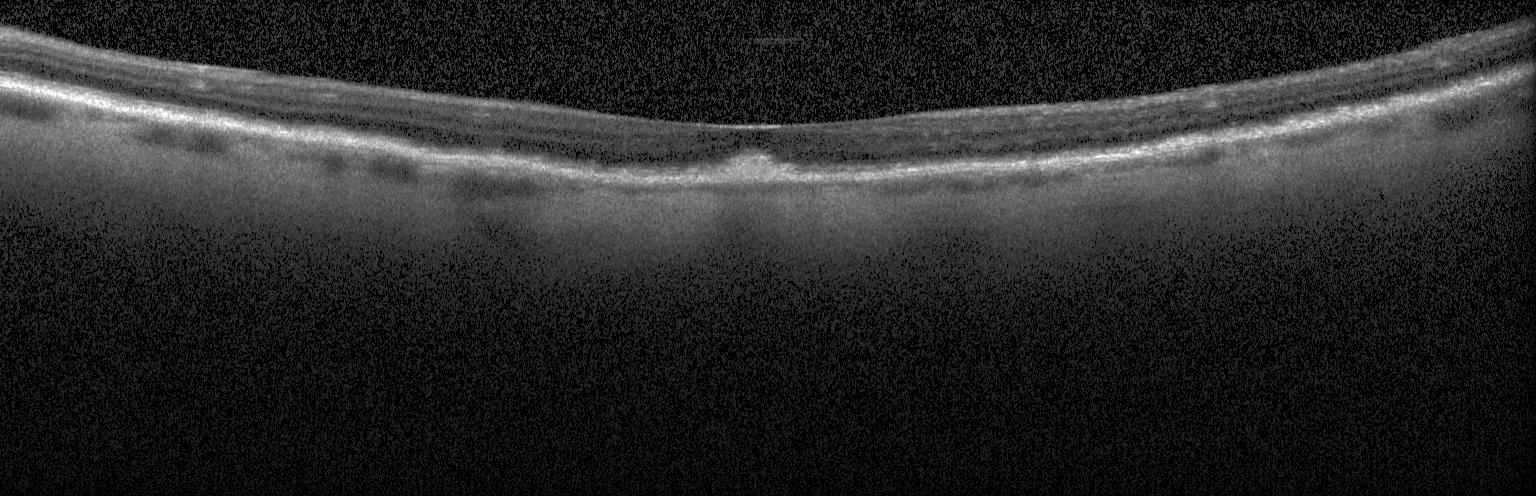
Finding: a choroidal neovascular membrane.